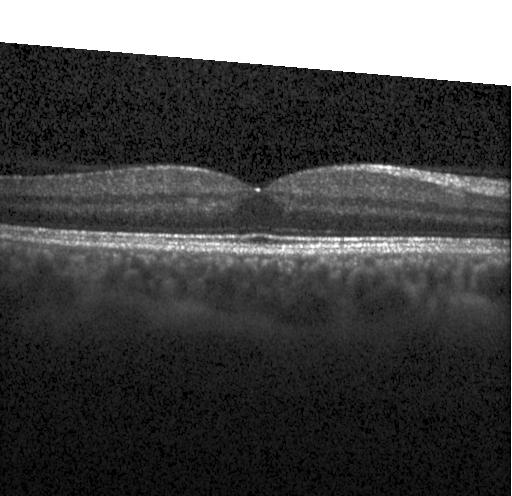
Fovea-centered. Spectral-domain OCT. Retinal OCT B-scan. Heidelberg Spectralis OCT system
Macular OCT: no CNV, no DME, and no drusen.